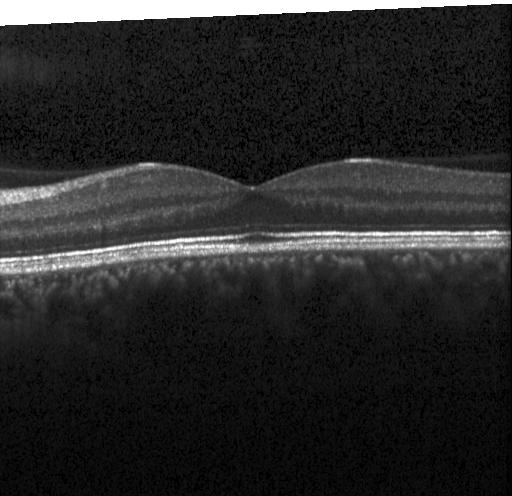

OCT line scan · spectral-domain optical coherence tomography · Heidelberg Spectralis OCT system — Diagnosis: no CNV, DME, or drusen.